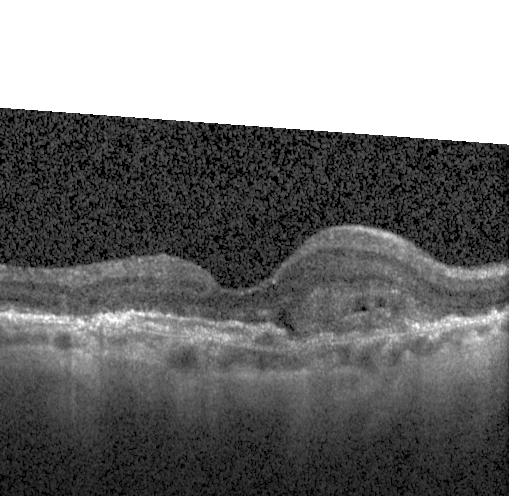

Retinal OCT cross-section, instrument: Heidelberg Spectralis.
Impression: choroidal neovascularization.